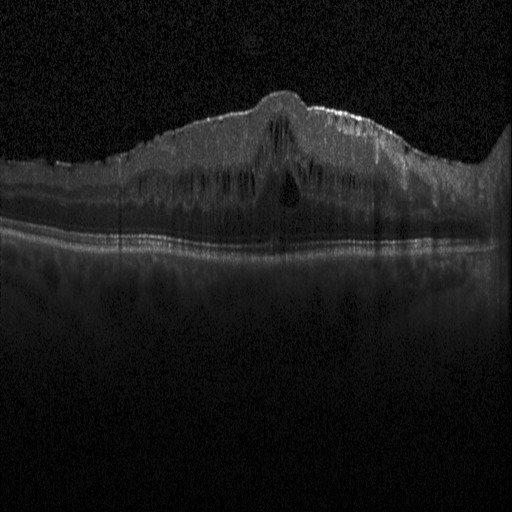
Spectral-domain optical coherence tomography. Heidelberg Spectralis. Fovea-centered. Retinal OCT cross-section — Finding: DME.